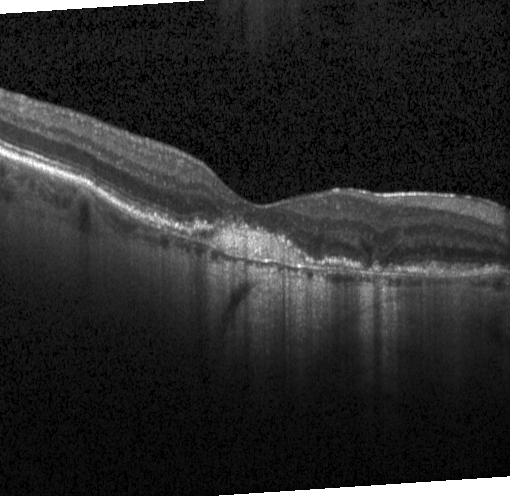 OCT B-scan showing a choroidal neovascular membrane.